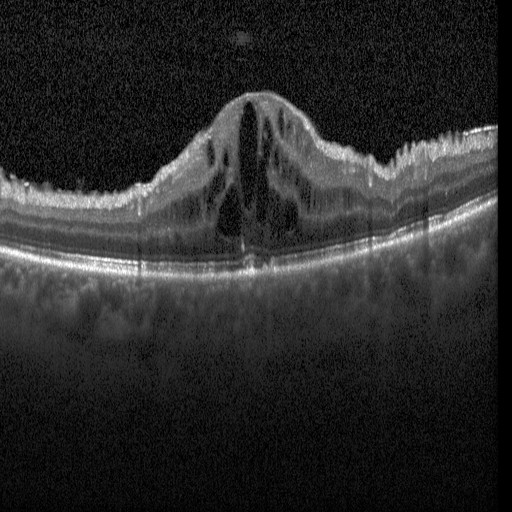 Optical coherence tomography scan. Spectral-domain OCT. Centered on the fovea. Heidelberg Spectralis OCT system. The scan shows diabetic macular edema.